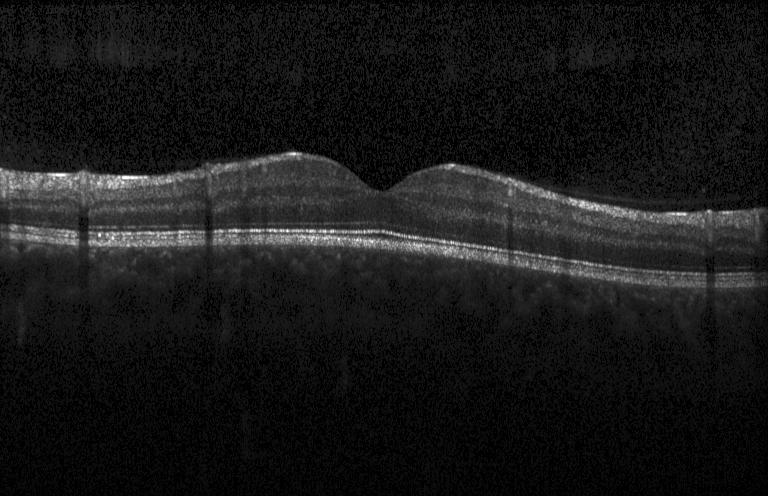
Fovea-centered. Acquired on a Heidelberg Spectralis. Spectral-domain OCT. OCT line scan.
Diagnosis: no CNV, DME, or drusen.